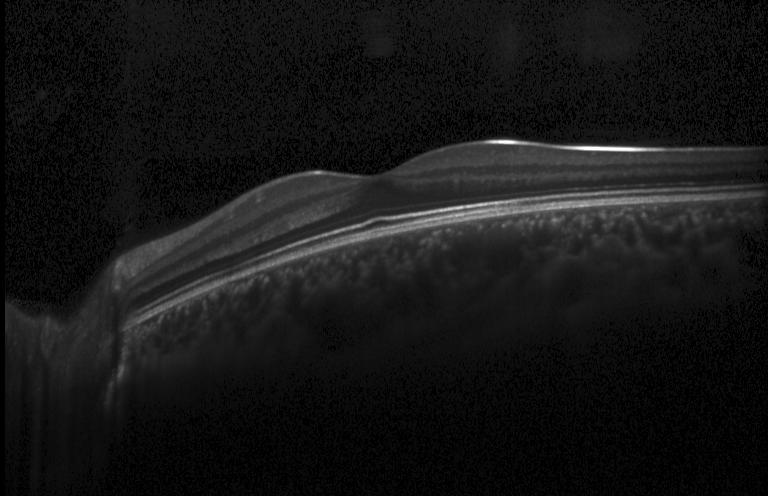
Macular OCT: no evidence of choroidal neovascularization, diabetic macular edema, or drusen.